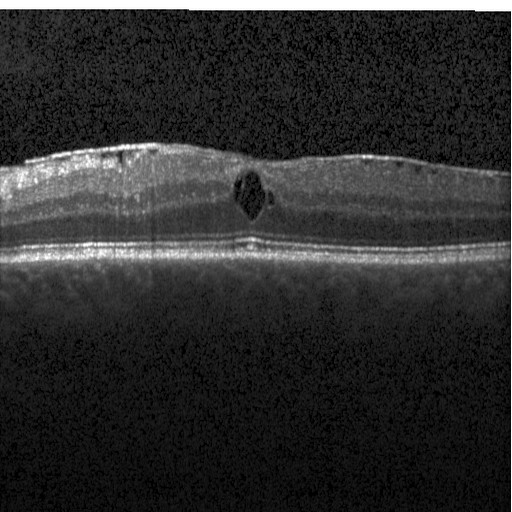
Finding: diabetic macular edema.